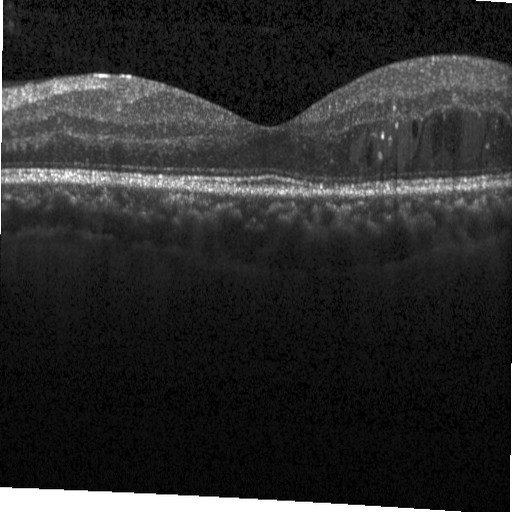
Optical coherence tomography B-scan · spectral-domain OCT.
The scan shows diabetic macular edema.